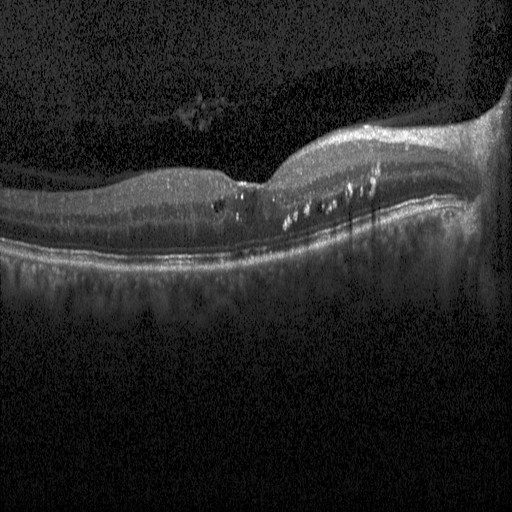
Instrument: Heidelberg Spectralis; retinal OCT cross-section. OCT finding: DME.